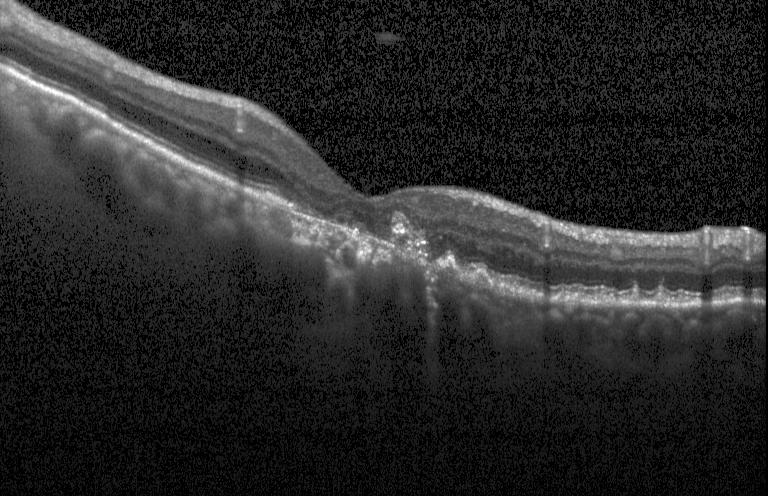 OCT line scan, SD-OCT, macular scan. Choroidal neovascularization (CNV).